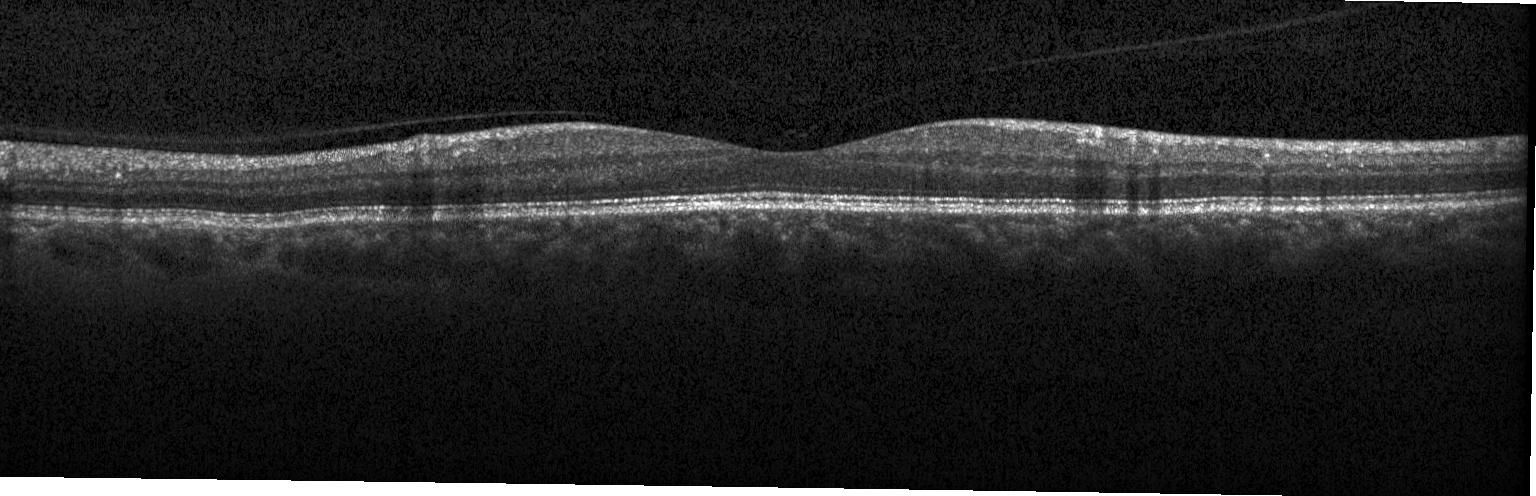 Fovea-centered. Optical coherence tomography scan. Heidelberg Spectralis OCT system. Spectral-domain optical coherence tomography
Finding: neither choroidal neovascularization, diabetic macular edema, nor drusen.